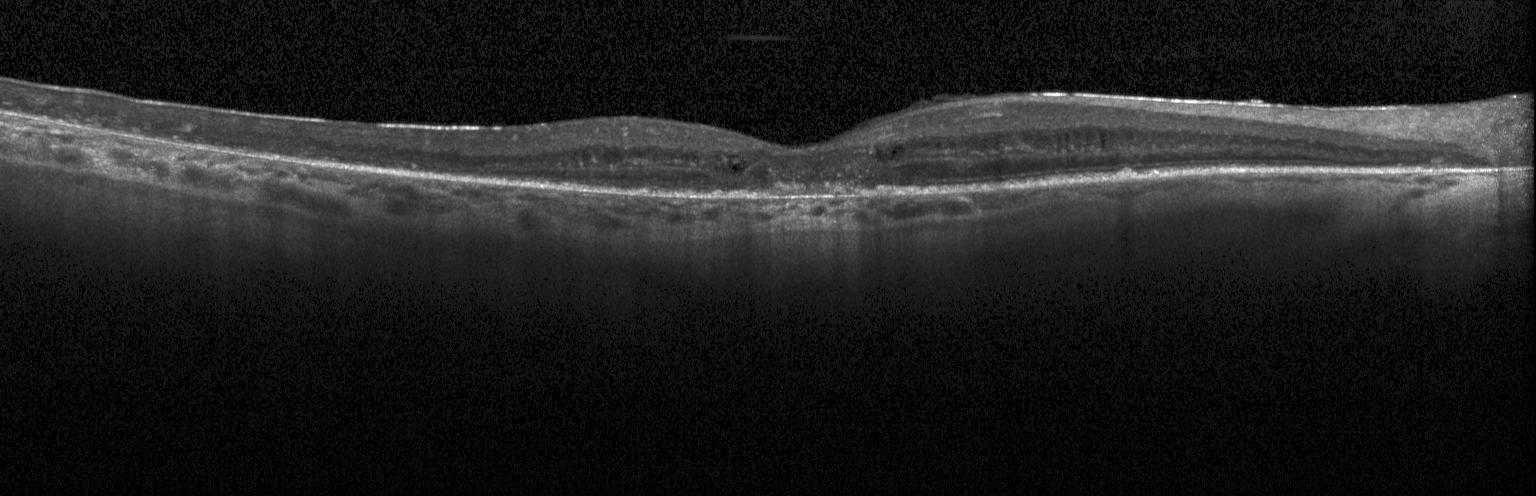 OCT scan showing a choroidal neovascular membrane.